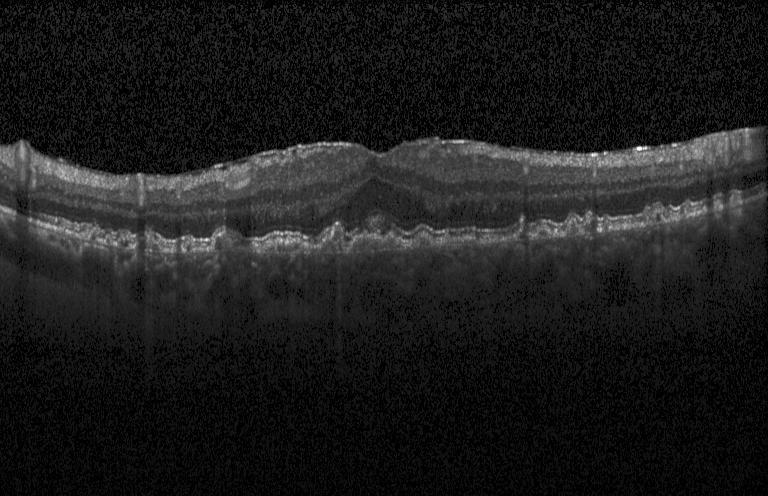 OCT B-scan — Finding: choroidal neovascularization (CNV).